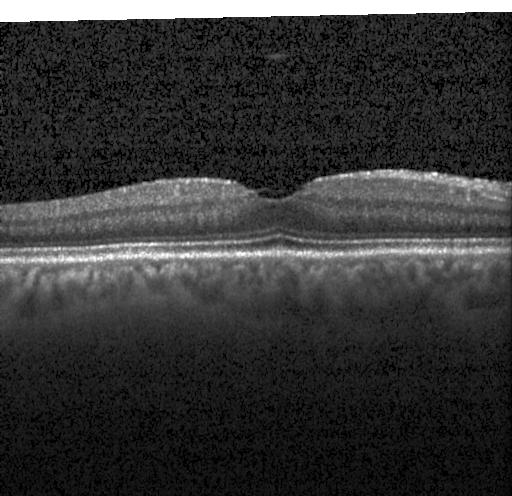 Optical coherence tomography scan, SD-OCT, horizontal scan through the fovea, Heidelberg Spectralis
Diagnosis: no choroidal neovascularization, no diabetic macular edema, and no drusen.